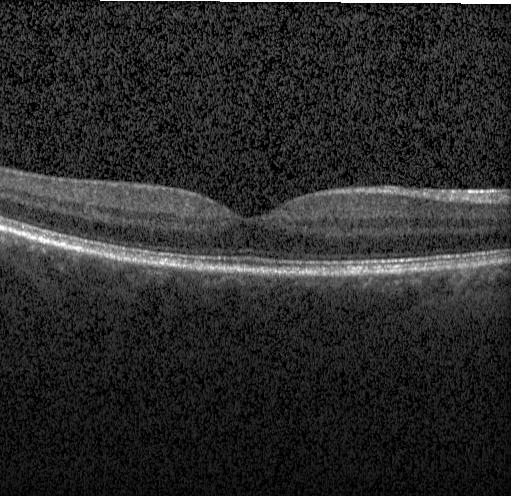
Macular scan; instrument: Heidelberg Spectralis; OCT B-scan; SD-OCT
Finding: no CNV, DME, or drusen.